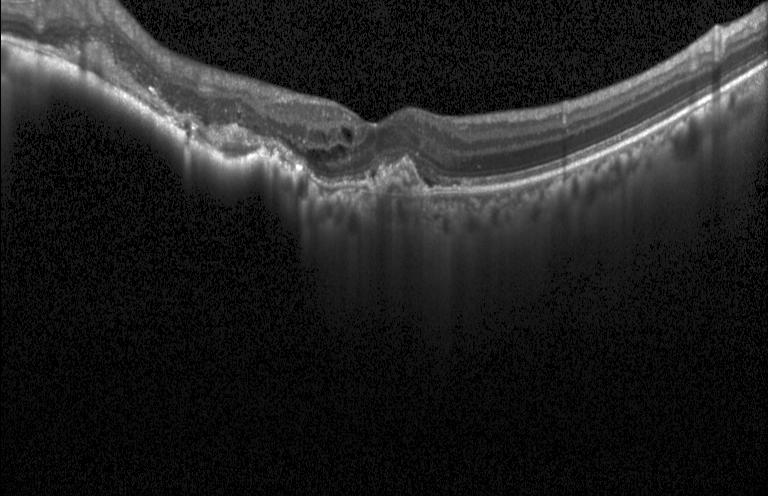
Macular OCT: a choroidal neovascular membrane.